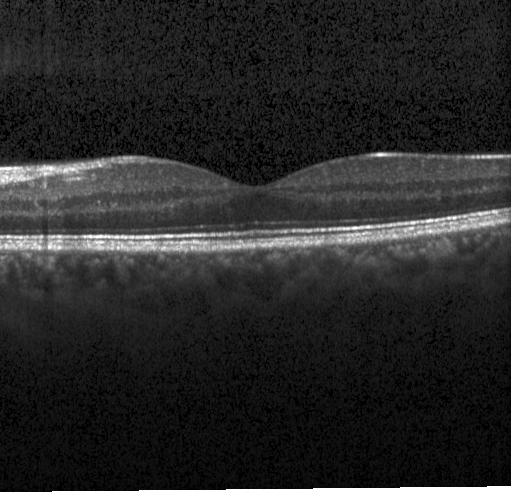 Spectral-domain OCT; horizontal scan through the fovea; retinal OCT B-scan
No choroidal neovascularization, no diabetic macular edema, and no drusen.